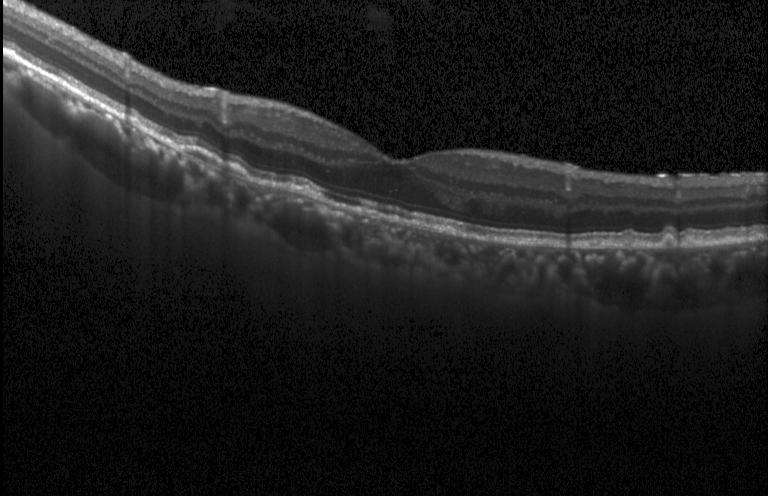
Heidelberg Spectralis OCT system; fovea-centered; retinal OCT B-scan; spectral-domain optical coherence tomography. Diagnosis: drusen.